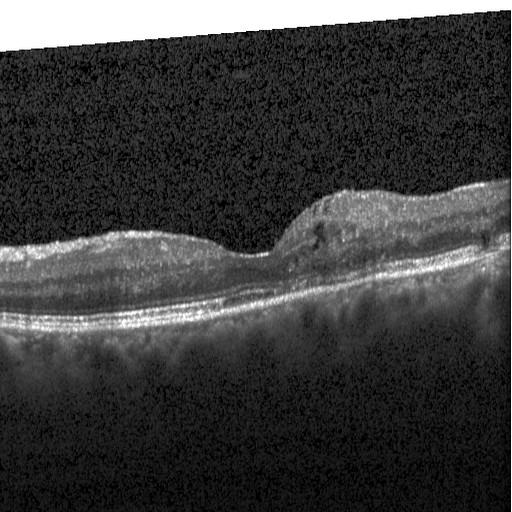
Centered on the fovea · retinal OCT cross-section.
Finding: DME.